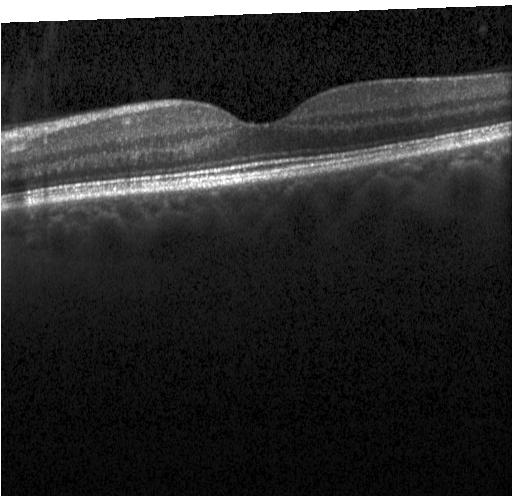

Heidelberg Spectralis OCT system, retinal OCT cross-section
Impression: no choroidal neovascularization, diabetic macular edema, or drusen.